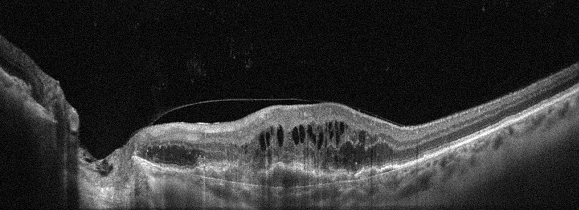
Oculus sinister, retinal OCT B-scan, through the macula
Assessment: age-related macular degeneration.